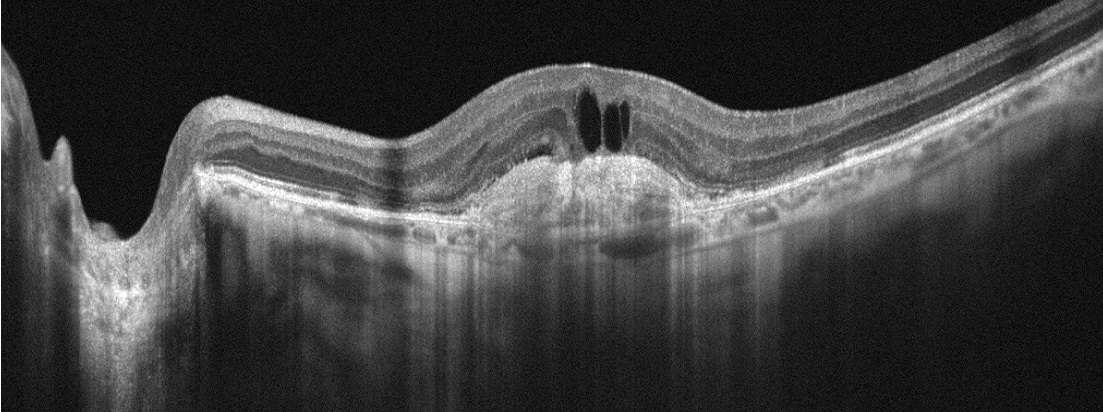 Retinal OCT cross-section.
Finding: age-related macular degeneration.